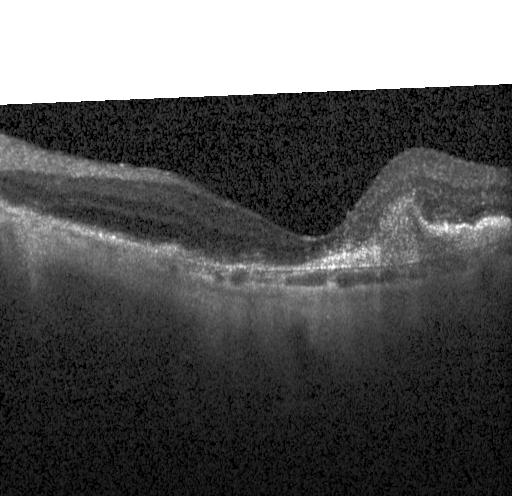 Retinal OCT B-scan, spectral-domain OCT. This B-scan demonstrates choroidal neovascularization (CNV).